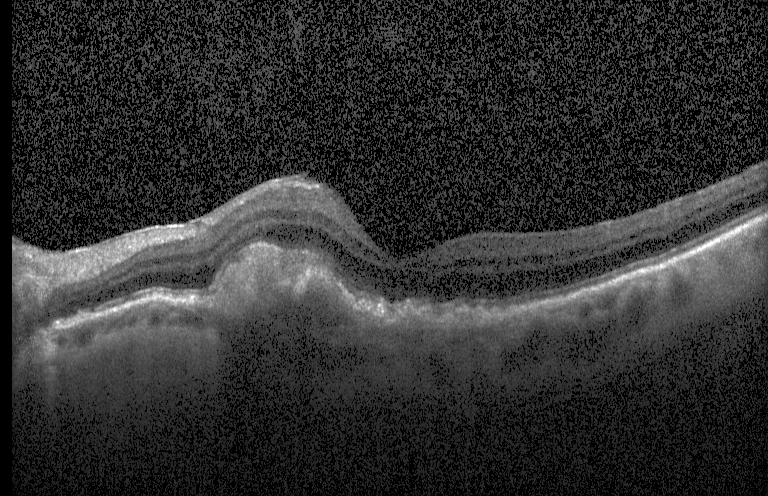
Through the macula; OCT line scan — Finding: a choroidal neovascular membrane.